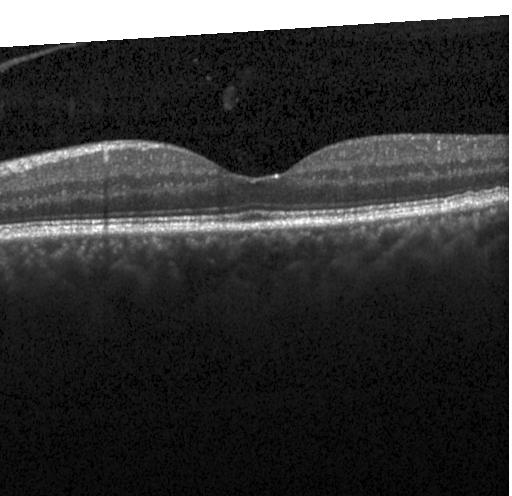
Through the macula; spectral-domain optical coherence tomography; retinal OCT cross-section.
Finding: neither CNV, DME, nor drusen.